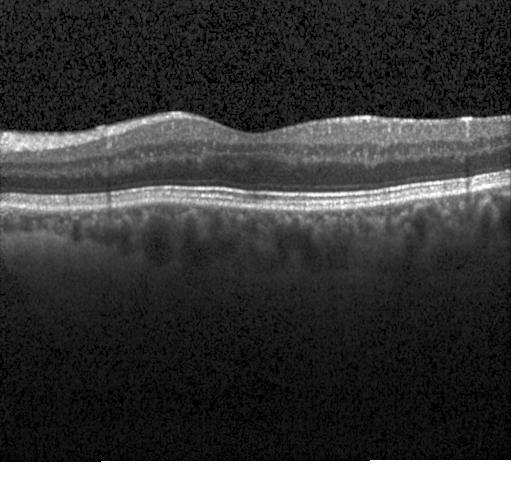 Impression: no CNV, no DME, and no drusen.